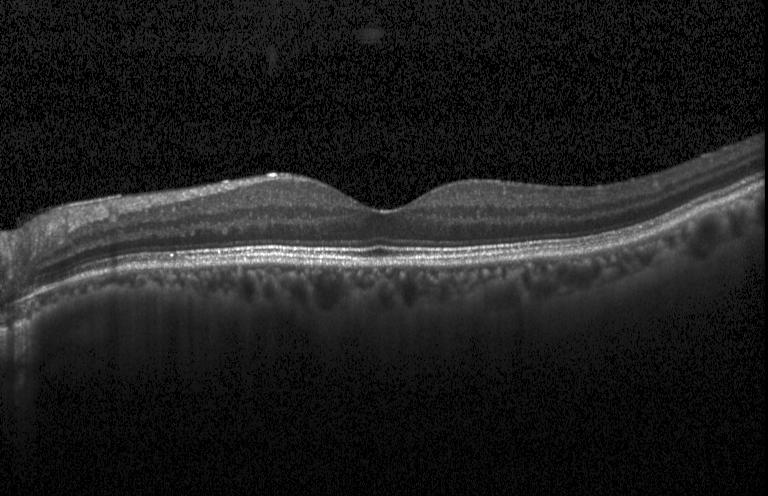

OCT B-scan showing neither choroidal neovascularization, diabetic macular edema, nor drusen.